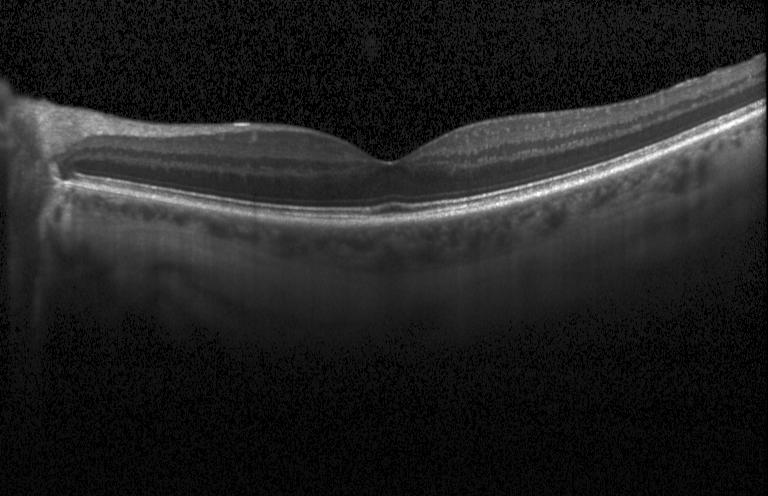 Spectral-domain optical coherence tomography; OCT line scan — Macular OCT: no CNV, no DME, and no drusen.